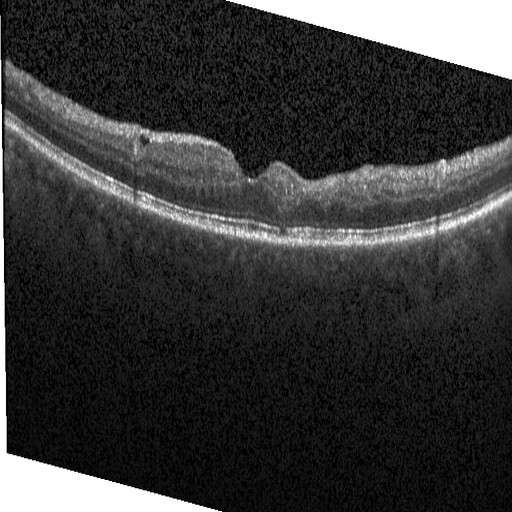
The scan shows diabetic macular edema.